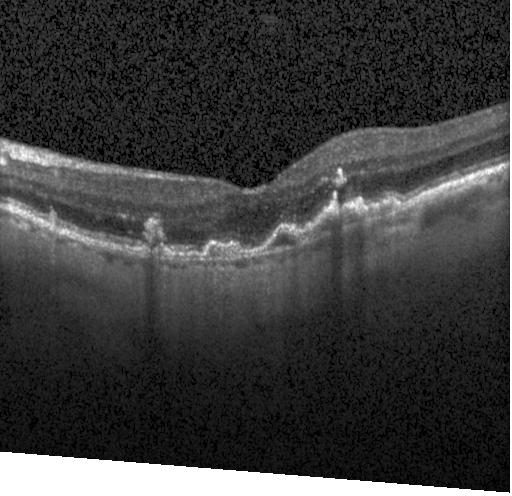 Assessment: a choroidal neovascular membrane.